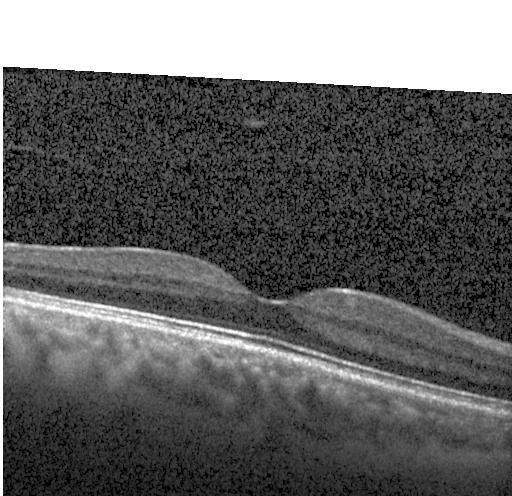 Retinal OCT cross-section. Spectral-domain OCT — Finding: neither choroidal neovascularization, diabetic macular edema, nor drusen.